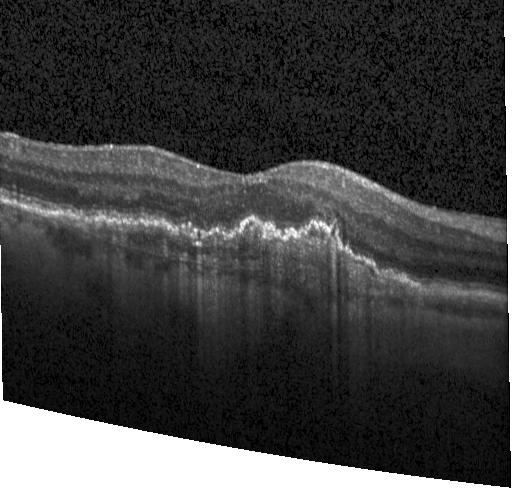
Optical coherence tomography scan.
Impression: CNV.